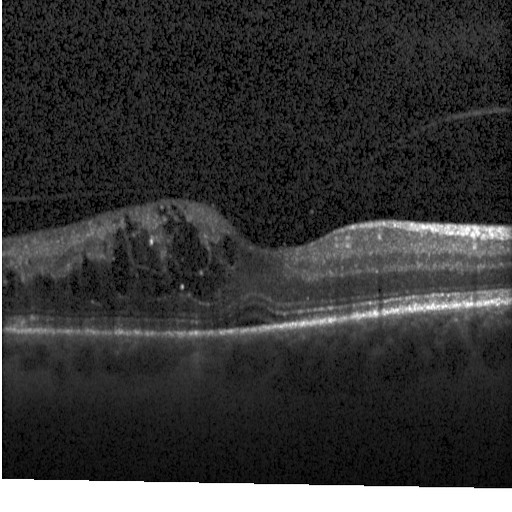 Macular scan; optical coherence tomography B-scan; spectral-domain optical coherence tomography
This B-scan demonstrates diabetic macular edema.